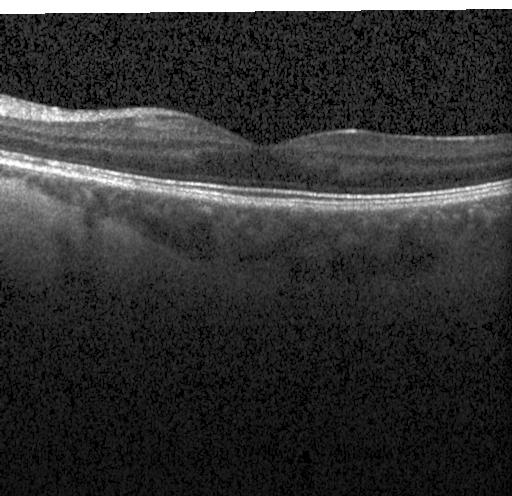 Retinal OCT B-scan — Diagnosis: no choroidal neovascularization, diabetic macular edema, or drusen.